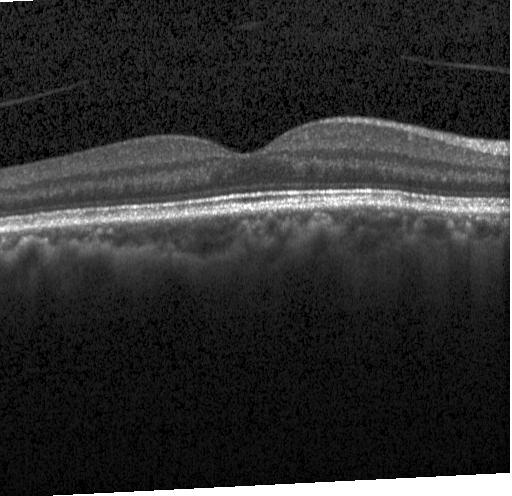
Acquired on a Heidelberg Spectralis · through the macula · OCT line scan · spectral-domain optical coherence tomography — Assessment: no CNV, no DME, and no drusen.